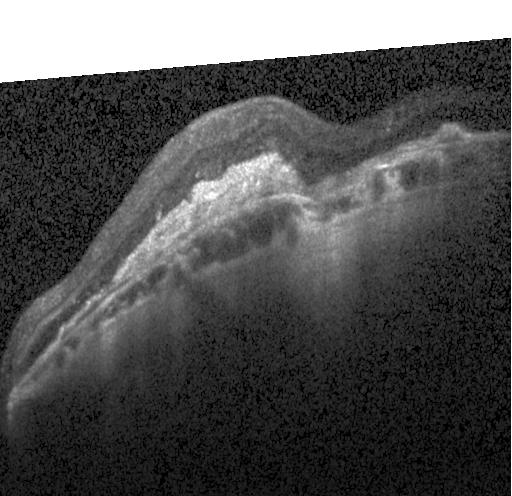 Dx: choroidal neovascularization.